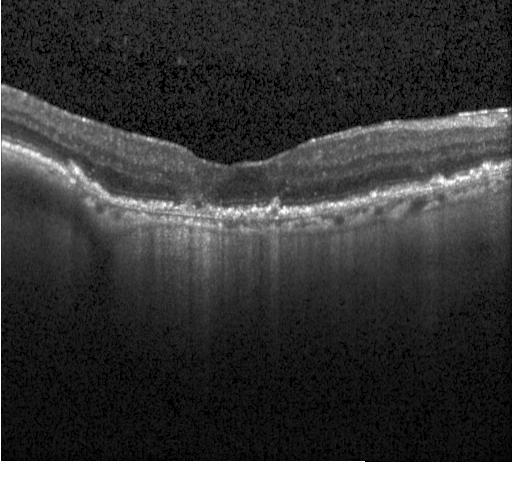 OCT finding: choroidal neovascularization (CNV).